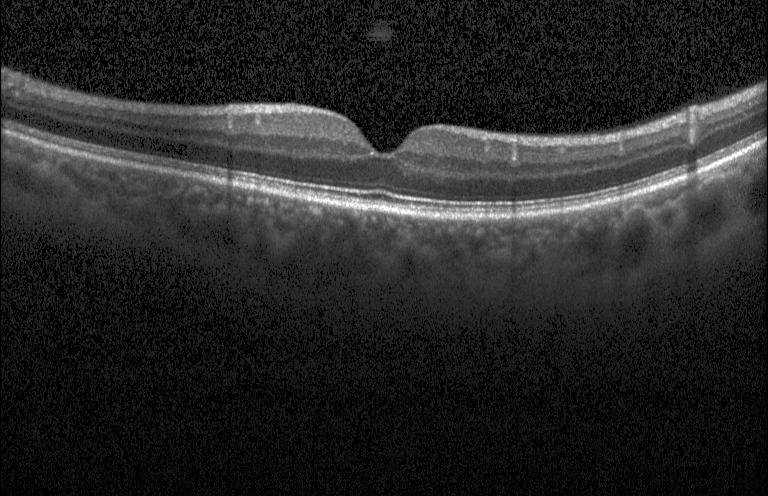

Spectral-domain OCT B-scan: no choroidal neovascularization, diabetic macular edema, or drusen.